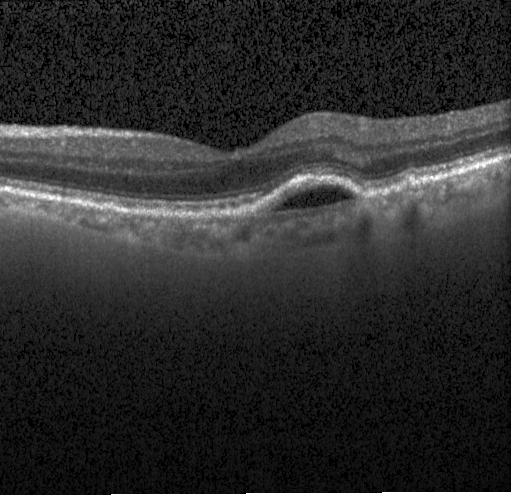 Acquired on a Heidelberg Spectralis, spectral-domain OCT, horizontal scan through the fovea, OCT line scan
Finding: choroidal neovascularization (CNV).